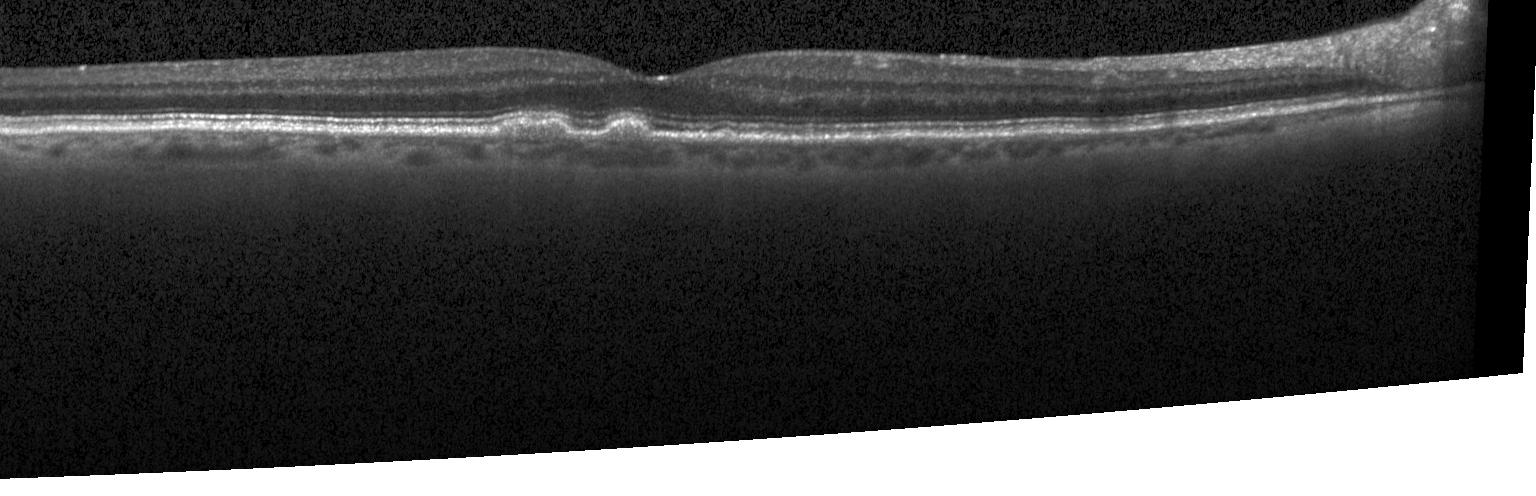
Macular scan; retinal OCT cross-section; acquired on a Heidelberg Spectralis. The scan shows sub-RPE drusenoid deposits.